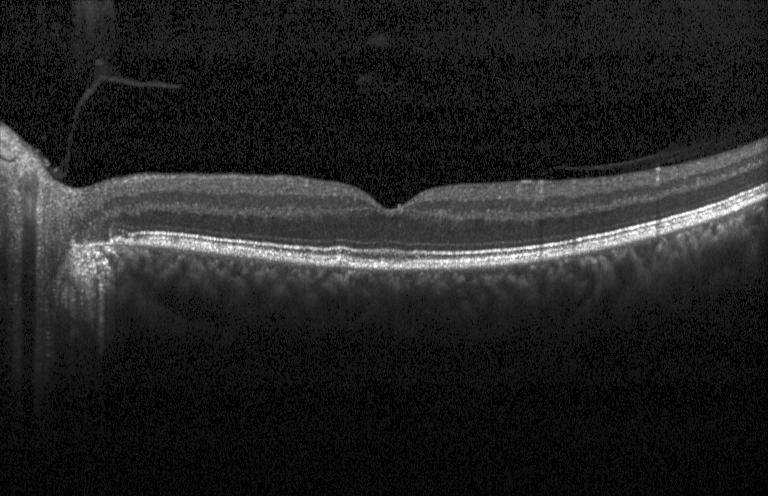

Spectral-domain OCT B-scan: sub-RPE drusenoid deposits.